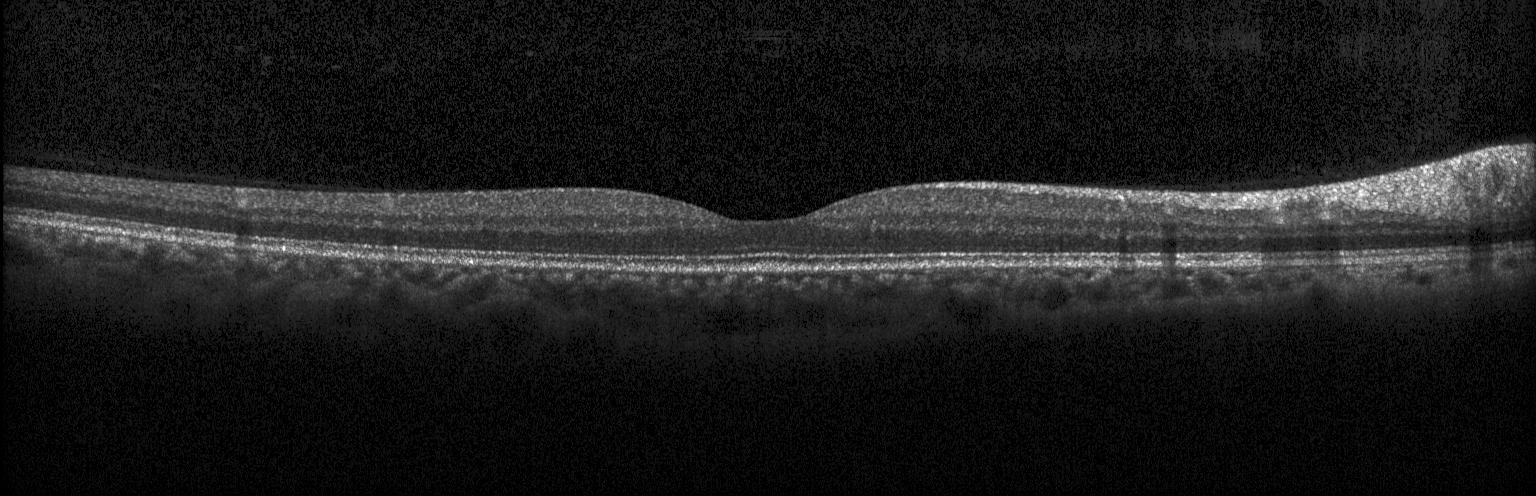
Fovea-centered, SD-OCT, retinal OCT B-scan — Diagnosis: no evidence of choroidal neovascularization, diabetic macular edema, or drusen.